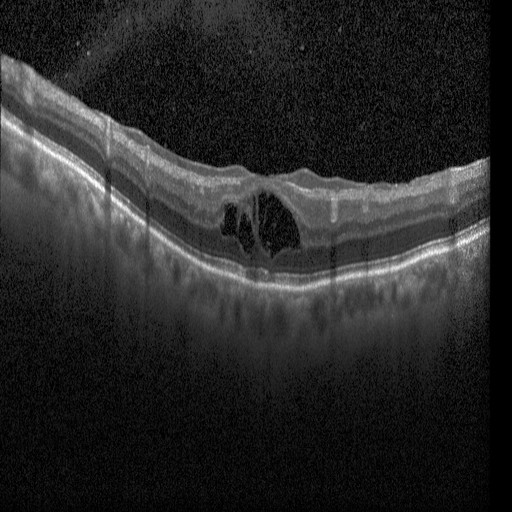
OCT finding: diabetic macular edema (DME).